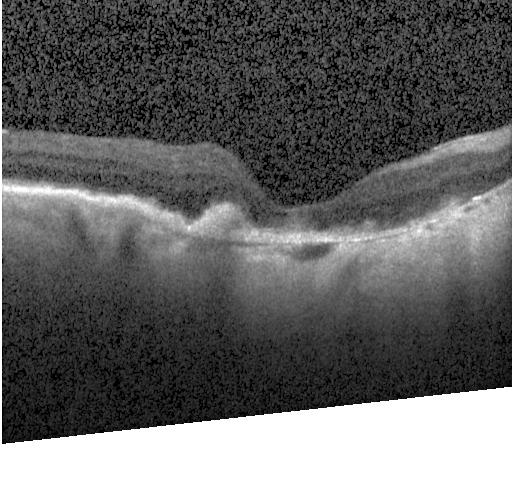

Assessment: a choroidal neovascular membrane.